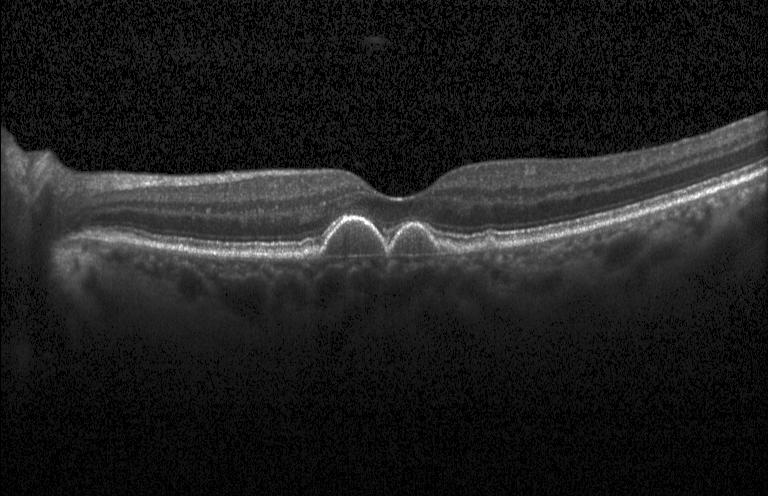
Optical coherence tomography B-scan; centered on the fovea; Heidelberg Spectralis.
Diagnosis: multiple drusen.